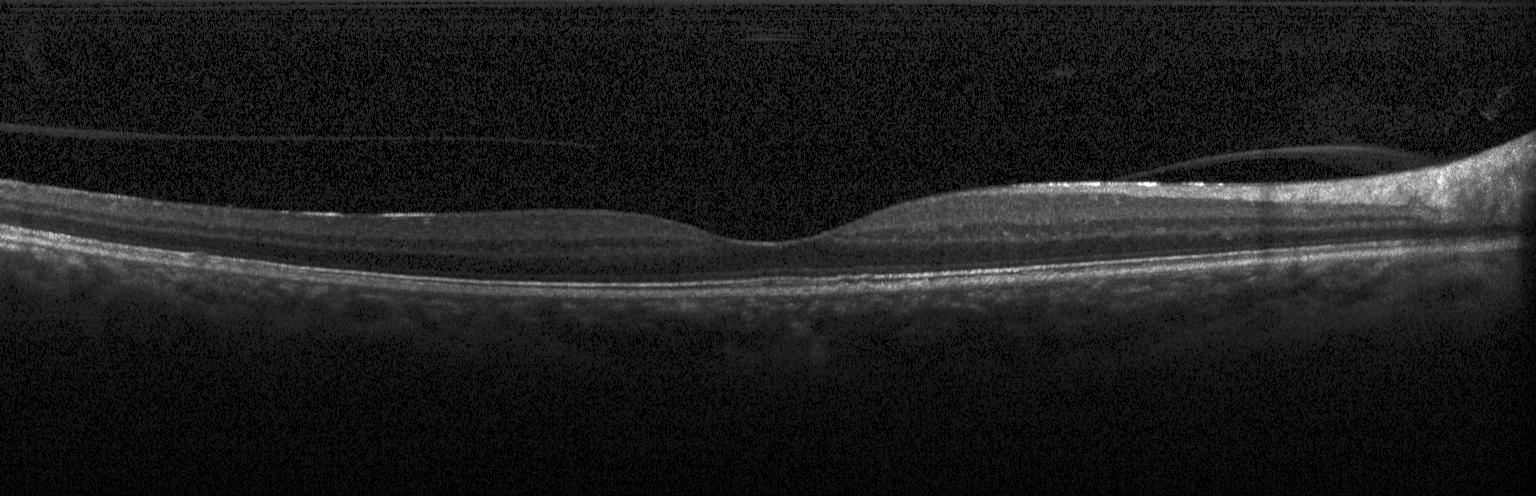

Fovea-centered · spectral-domain OCT · OCT line scan. OCT finding: neither choroidal neovascularization, diabetic macular edema, nor drusen.